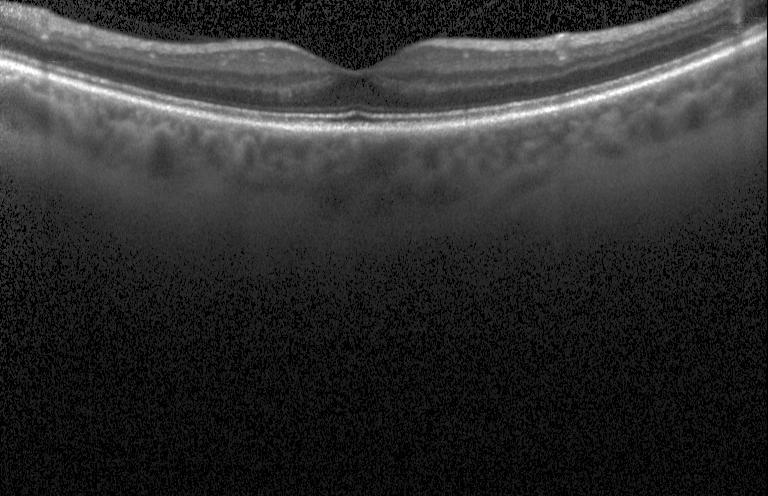
Retinal OCT cross-section. Finding: neither choroidal neovascularization, diabetic macular edema, nor drusen.